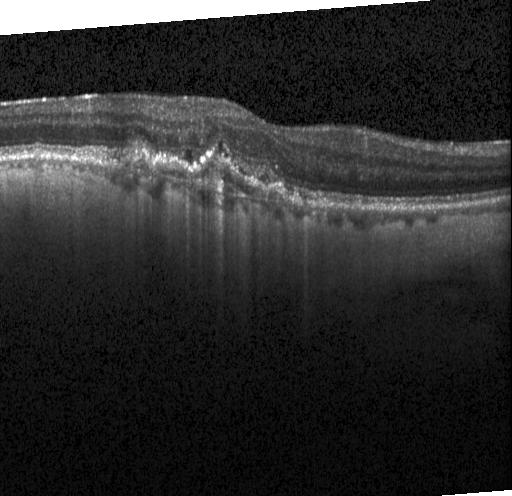
Optical coherence tomography B-scan.
Assessment: a choroidal neovascular membrane.